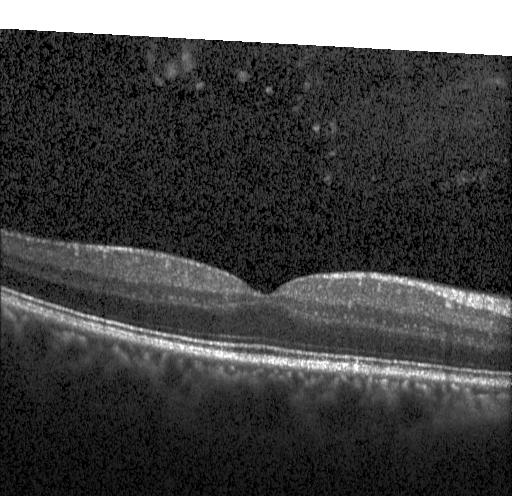 SD-OCT. Retinal OCT B-scan. Heidelberg Spectralis OCT system
The scan shows neither choroidal neovascularization, diabetic macular edema, nor drusen.